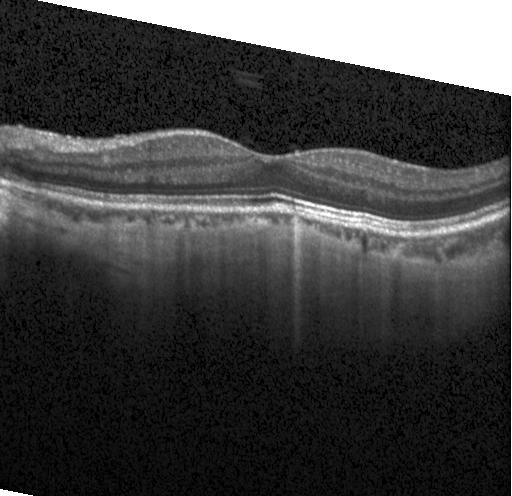
OCT B-scan · Heidelberg Spectralis · spectral-domain optical coherence tomography — Diagnosis: no CNV, DME, or drusen.